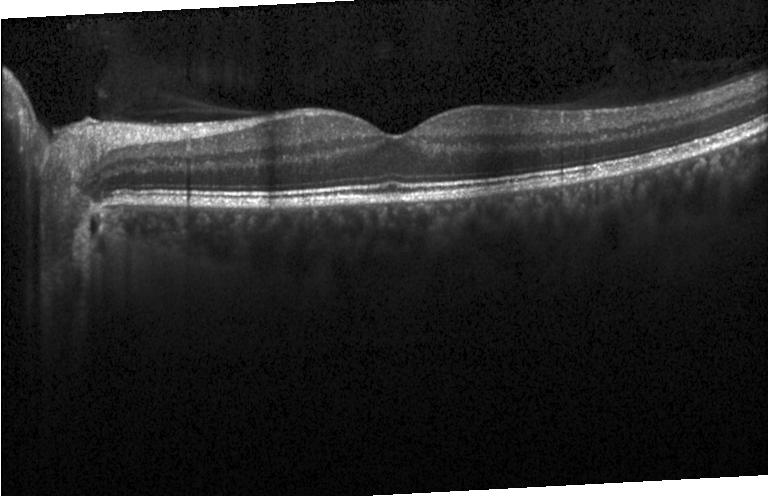
Through the macula. Spectral-domain OCT. OCT B-scan. Acquired on a Heidelberg Spectralis — Macular OCT: neither CNV, DME, nor drusen.